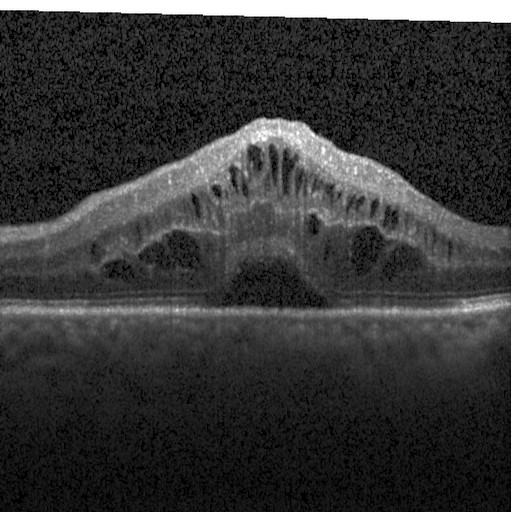 Macular OCT: diabetic macular edema.